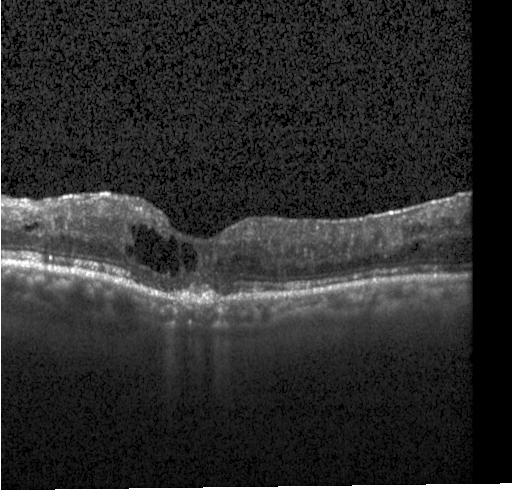

Macular scan · OCT line scan.
Impression: CNV.